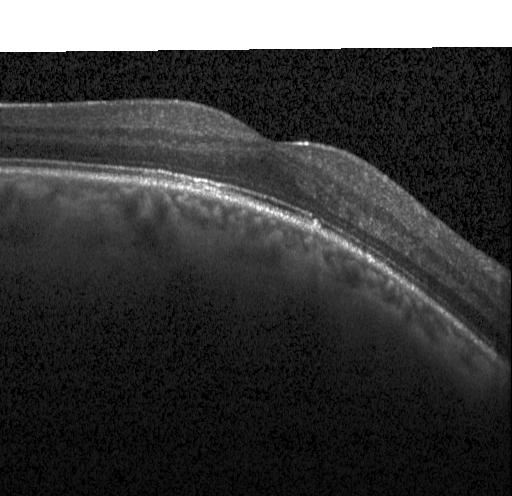
Heidelberg Spectralis. OCT line scan. Horizontal scan through the fovea
This B-scan demonstrates no evidence of CNV, DME, or drusen.